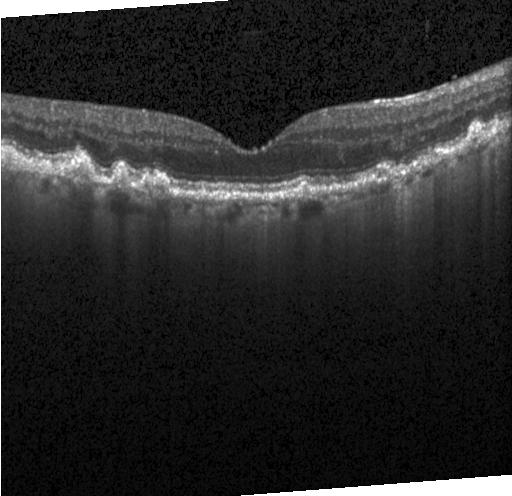
OCT B-scan. Fovea-centered. Acquired on a Heidelberg Spectralis. Spectral-domain OCT.
Sub-RPE drusenoid deposits.